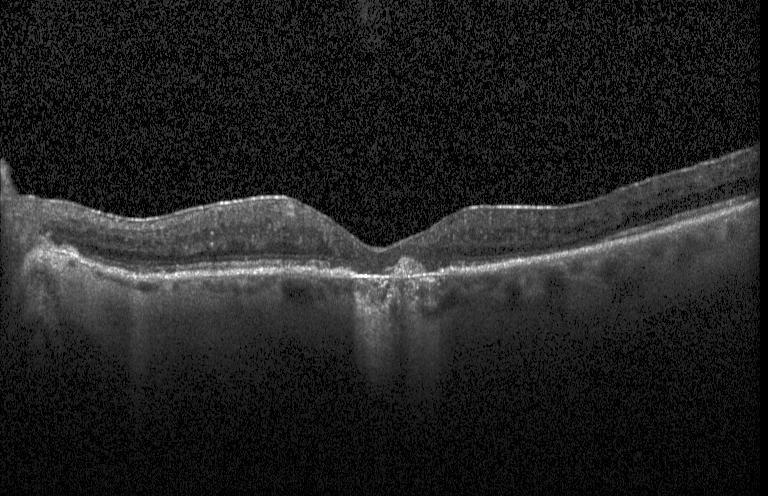
Fovea-centered, acquired on a Heidelberg Spectralis, retinal OCT B-scan.
Impression: a choroidal neovascular membrane.